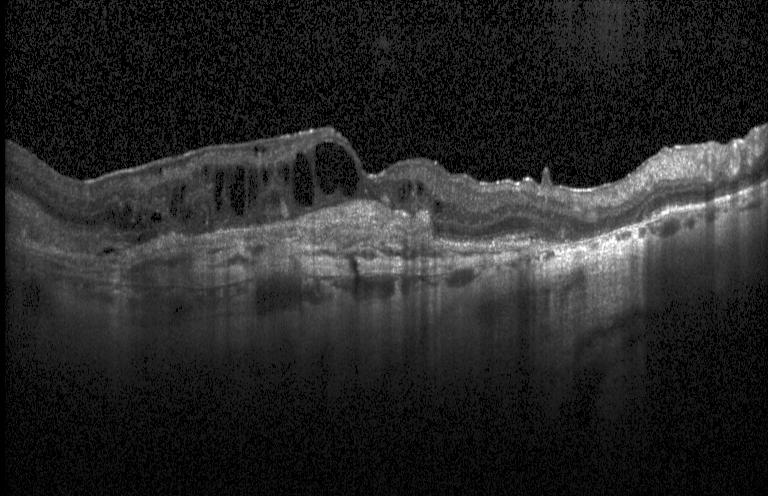

Retinal OCT cross-section showing choroidal neovascularization.